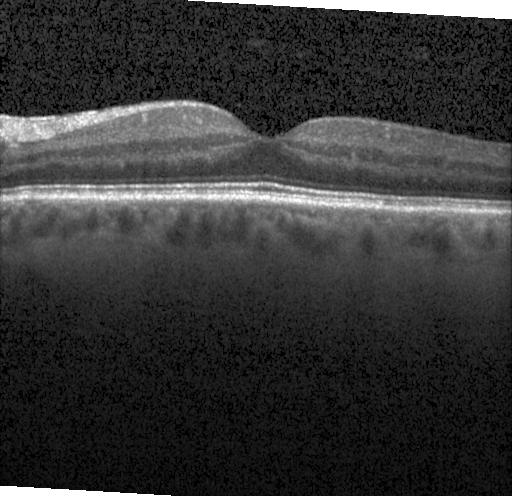
SD-OCT; optical coherence tomography B-scan — The scan shows neither choroidal neovascularization, diabetic macular edema, nor drusen.